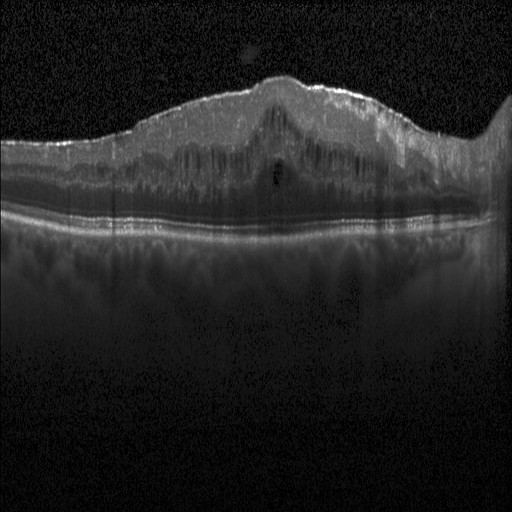

This B-scan demonstrates diabetic macular edema.